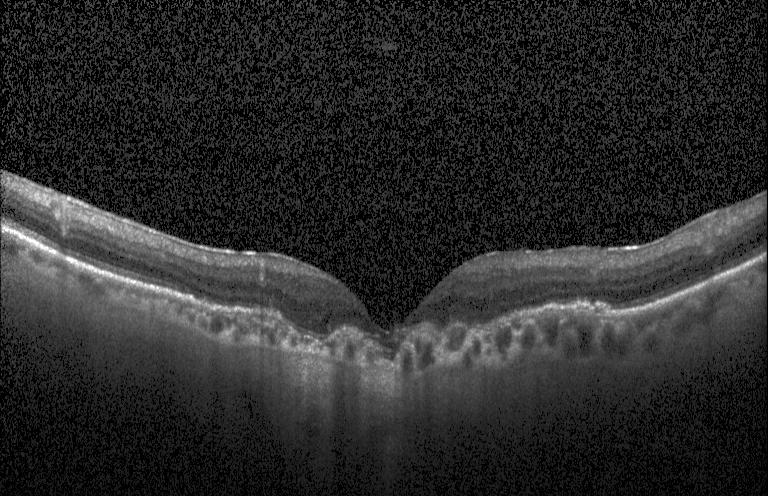

Diagnosis: a choroidal neovascular membrane.